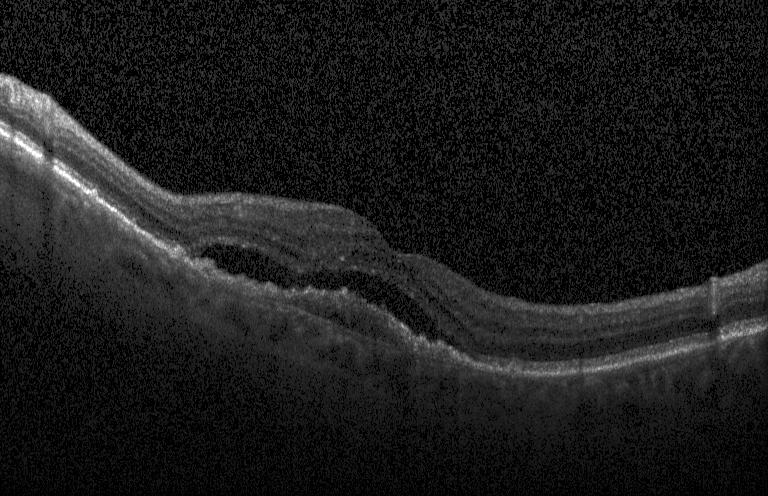
Macular OCT: choroidal neovascularization.